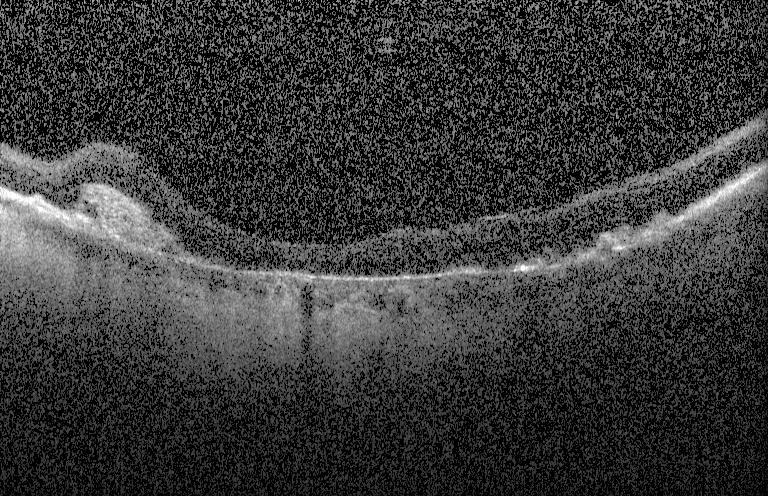

CNV.